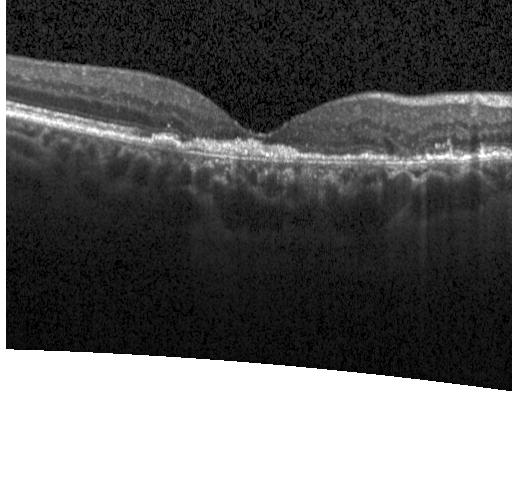
Heidelberg Spectralis OCT system; OCT B-scan. Assessment: a choroidal neovascular membrane.